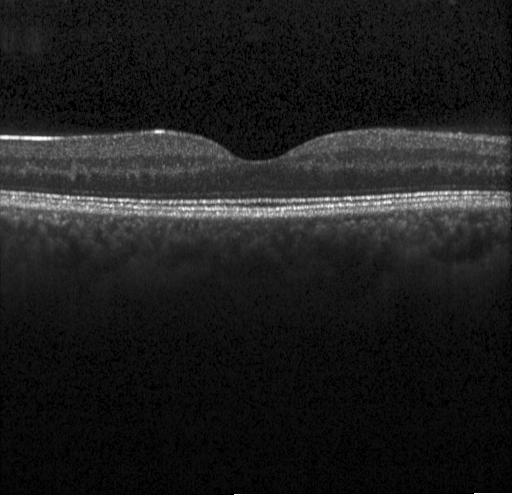

Acquired on a Heidelberg Spectralis; OCT B-scan; SD-OCT; fovea-centered. Impression: no CNV, DME, or drusen.